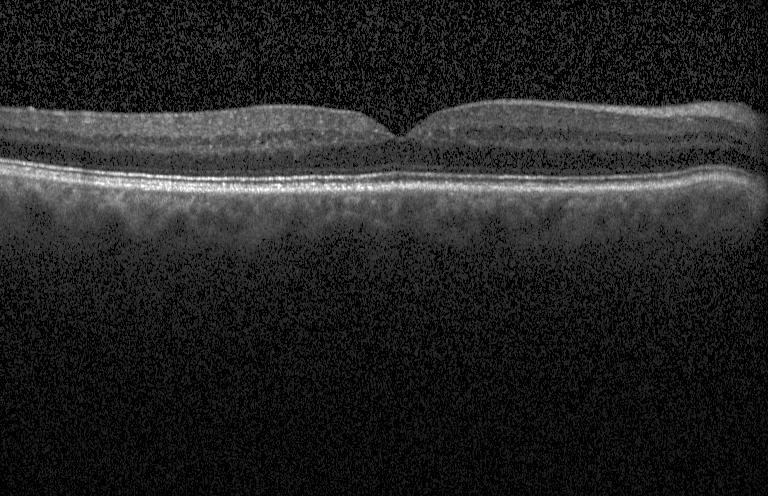 Retinal OCT cross-section. No choroidal neovascularization, no diabetic macular edema, and no drusen.